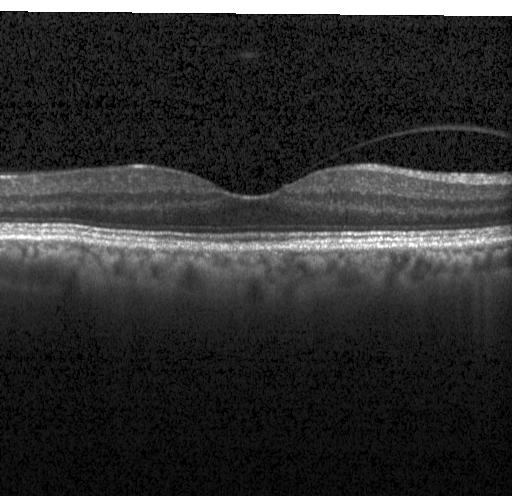
SD-OCT · OCT line scan. This B-scan demonstrates no evidence of choroidal neovascularization, diabetic macular edema, or drusen.